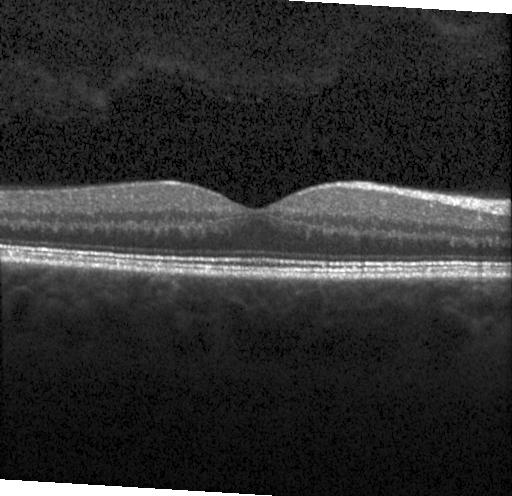 OCT B-scan
Impression: no choroidal neovascularization, diabetic macular edema, or drusen.